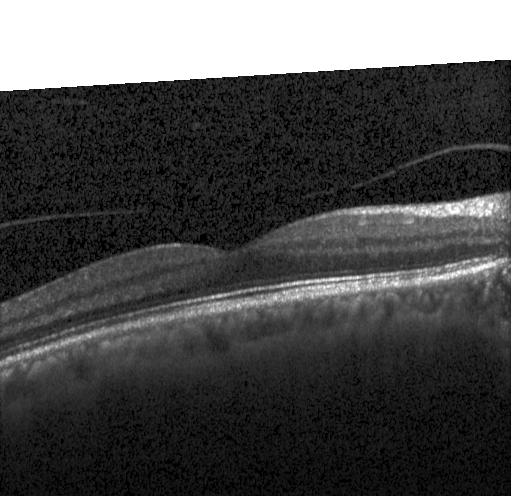
Macular OCT: neither CNV, DME, nor drusen.